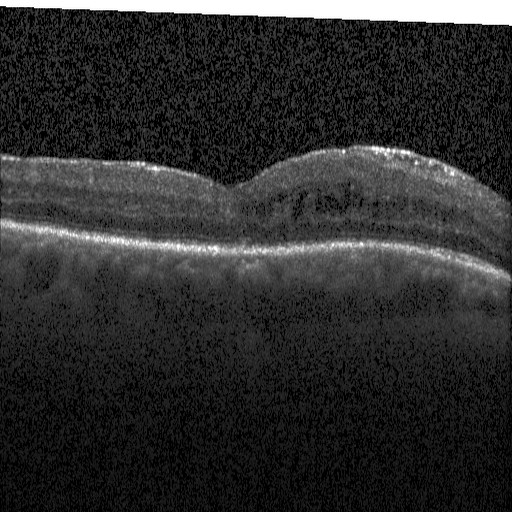 Fovea-centered. Retinal OCT B-scan. Spectral-domain OCT.
Macular OCT: diabetic macular edema.